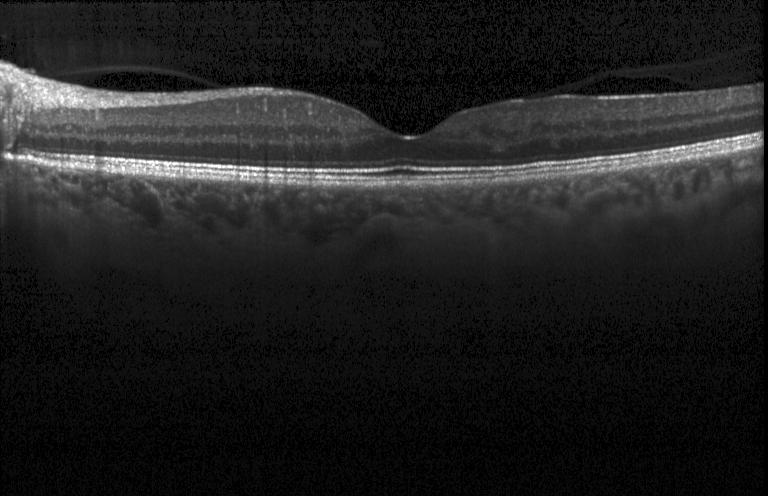 Diagnosis: no choroidal neovascularization, diabetic macular edema, or drusen.